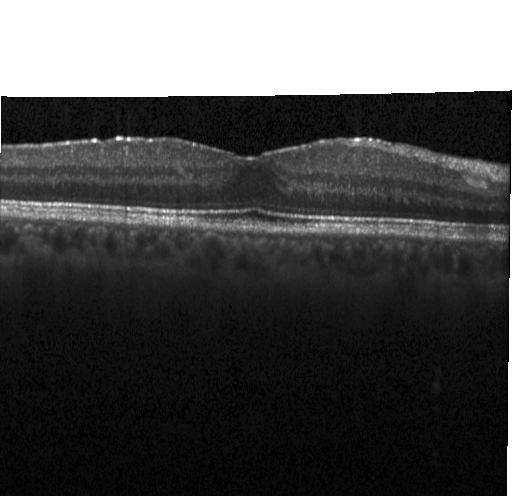

Through the macula, OCT B-scan.
Macular OCT: no evidence of choroidal neovascularization, diabetic macular edema, or drusen.